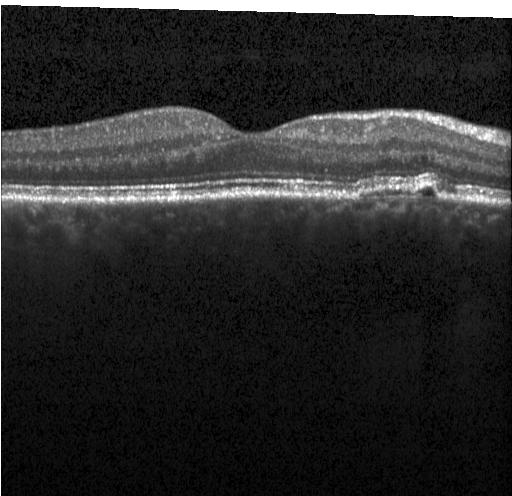

This B-scan demonstrates a choroidal neovascular membrane.